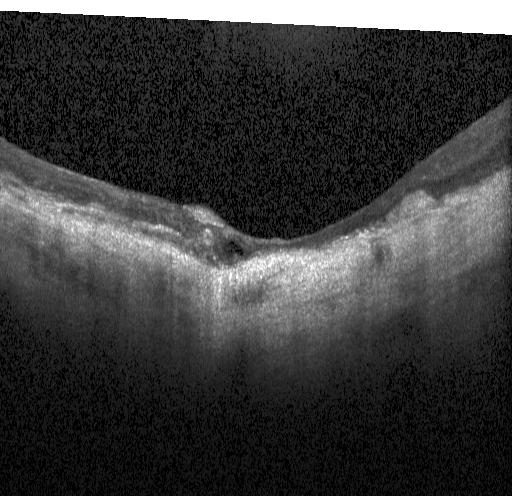

OCT B-scan — This B-scan demonstrates a choroidal neovascular membrane.